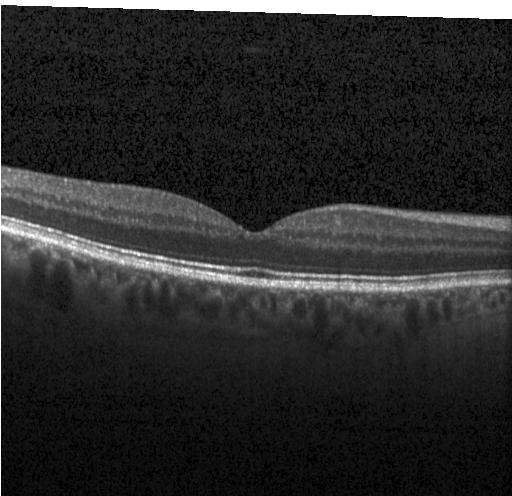
OCT finding: no choroidal neovascularization, diabetic macular edema, or drusen.